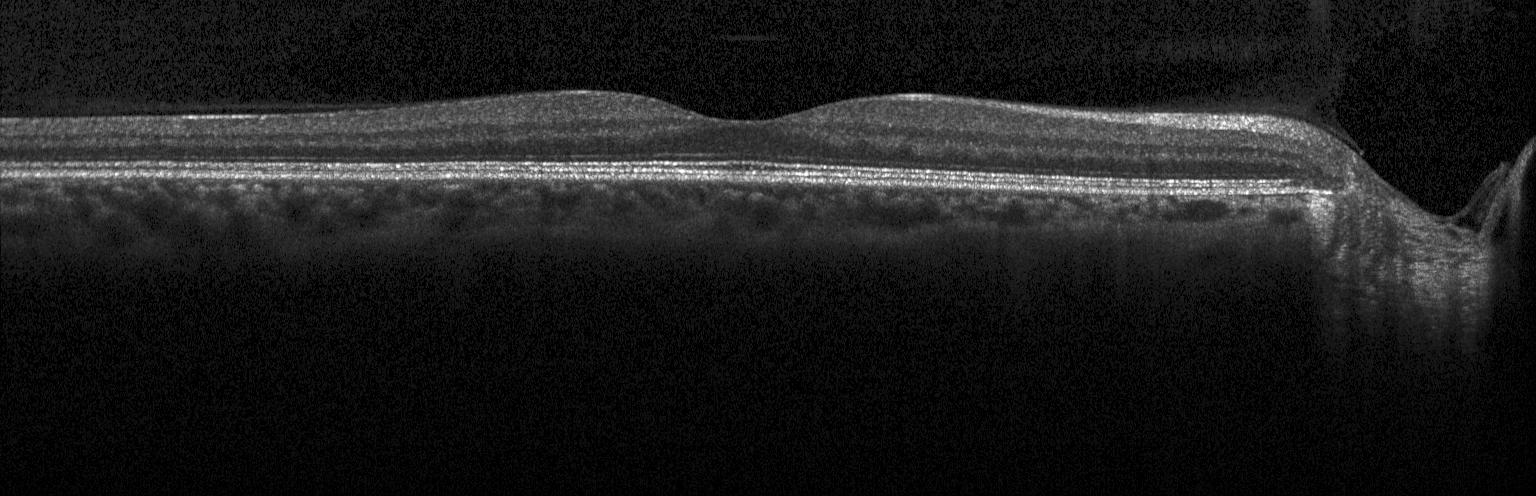 Impression: neither choroidal neovascularization, diabetic macular edema, nor drusen.